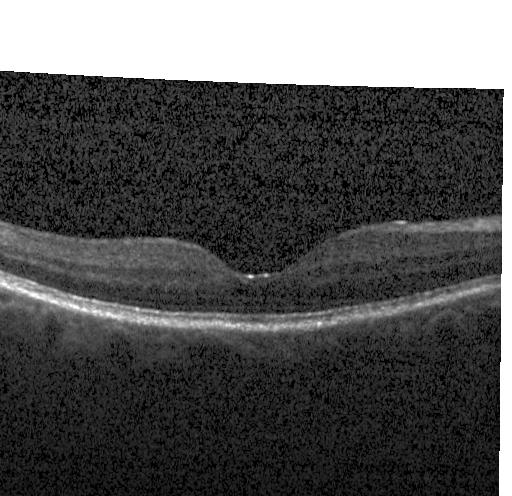

Diagnosis: no CNV, DME, or drusen.